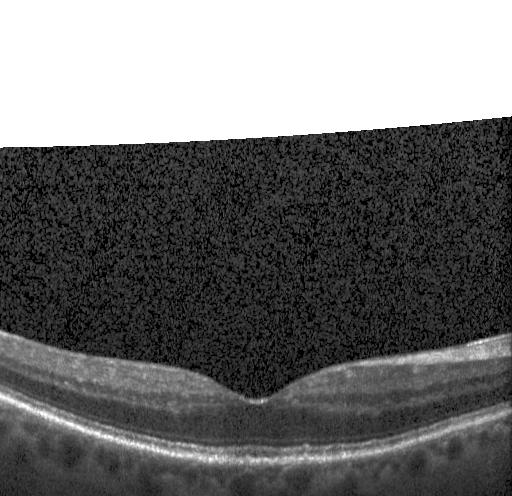

Acquired on a Heidelberg Spectralis; fovea-centered; spectral-domain OCT; retinal OCT B-scan. This B-scan demonstrates no CNV, DME, or drusen.